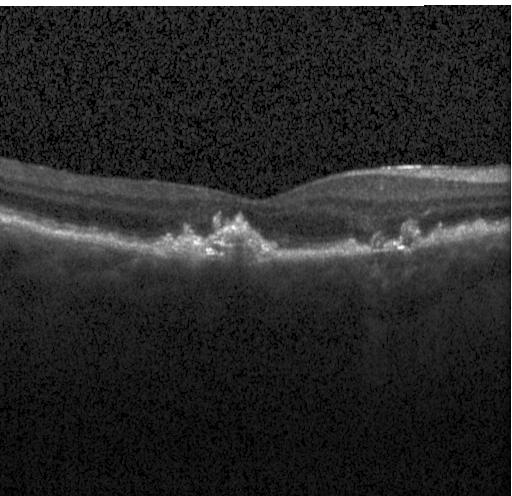 Spectral-domain OCT B-scan: CNV.